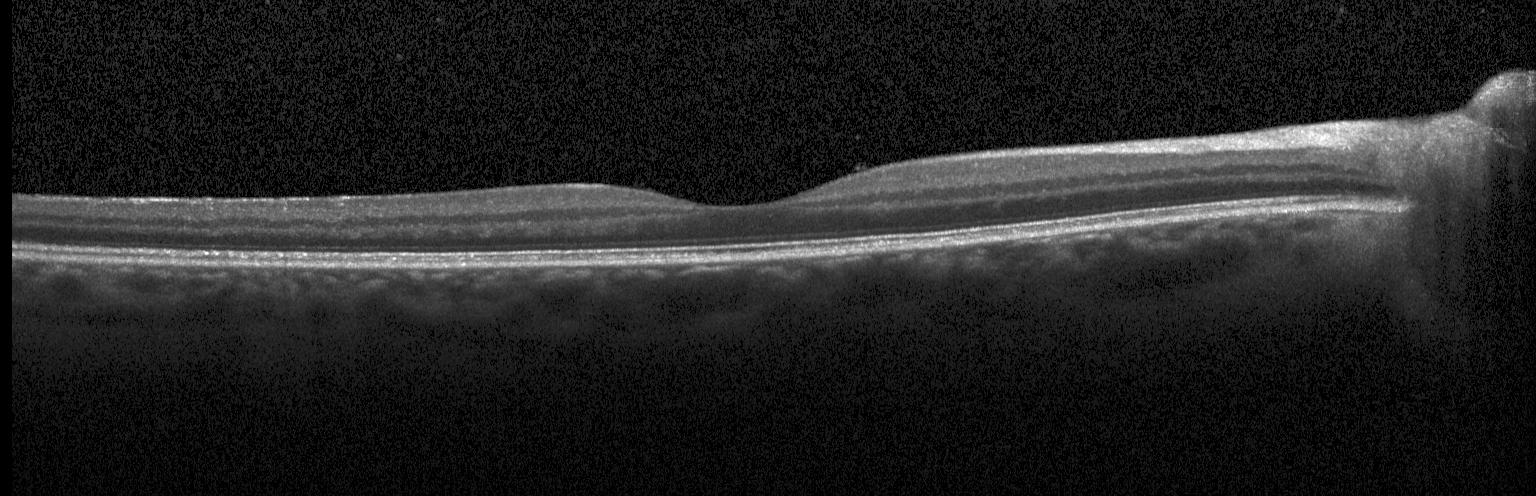
Fovea-centered · SD-OCT · OCT B-scan. Assessment: no CNV, no DME, and no drusen.